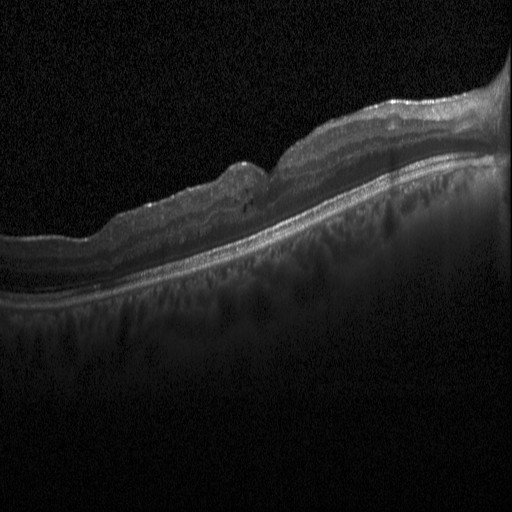 Through the macula, OCT B-scan — Assessment: diabetic macular edema (DME).